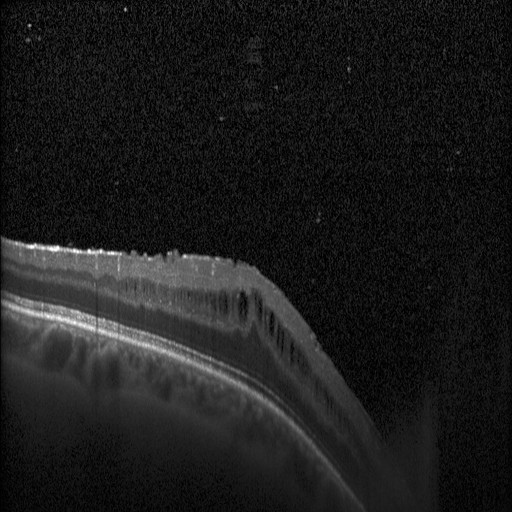
DME.